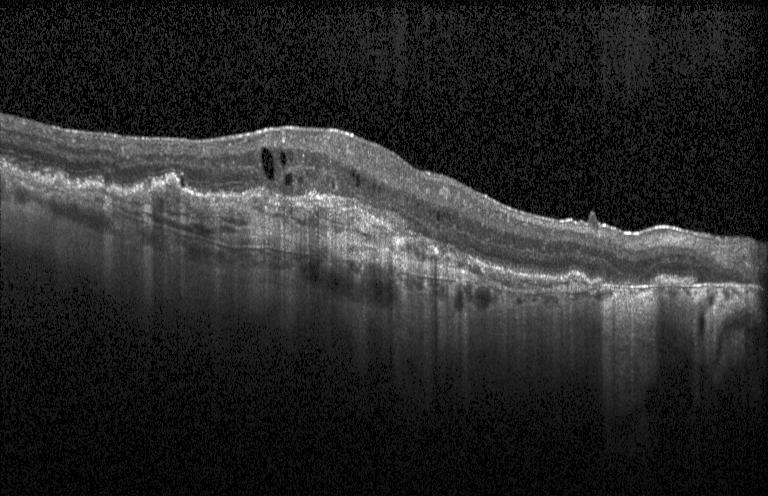
Spectral-domain OCT, optical coherence tomography scan.
Diagnosis: a choroidal neovascular membrane.